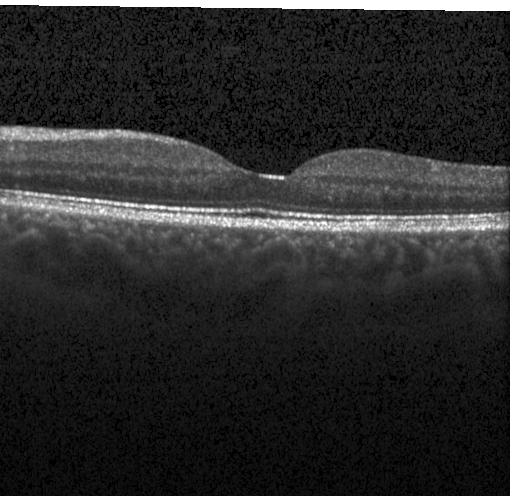

Fovea-centered, SD-OCT, instrument: Heidelberg Spectralis, OCT B-scan
Finding: no choroidal neovascularization, no diabetic macular edema, and no drusen.